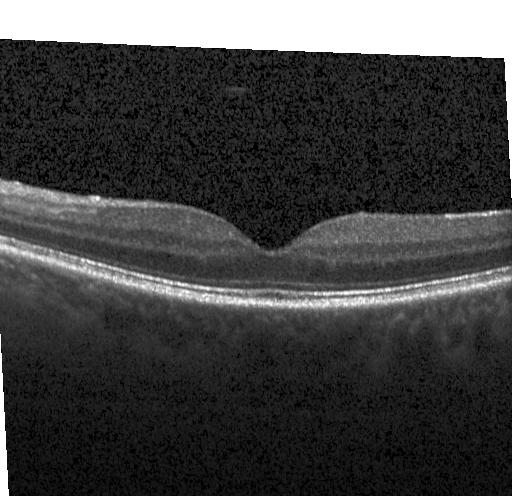
Spectral-domain optical coherence tomography · OCT B-scan
Finding: no choroidal neovascularization, diabetic macular edema, or drusen.